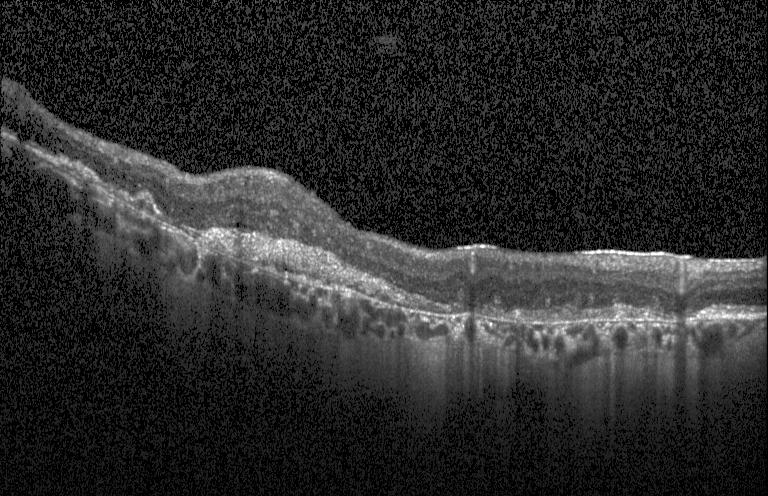

Heidelberg Spectralis OCT system. OCT line scan. SD-OCT. Macular scan
Diagnosis: choroidal neovascularization (CNV).